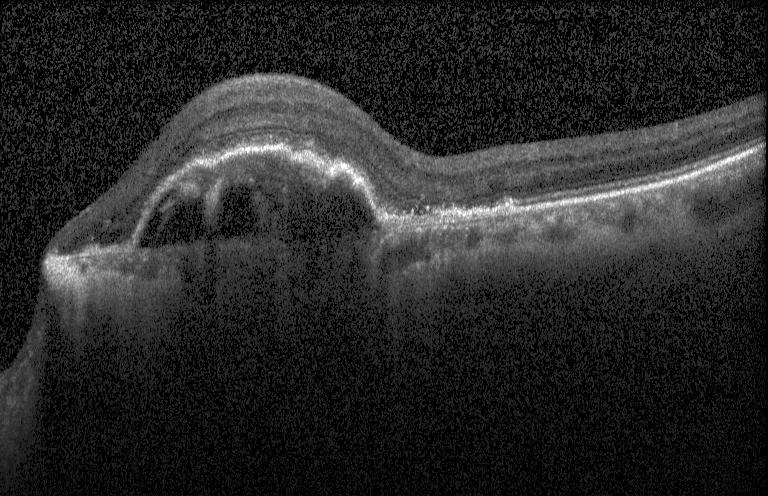

OCT B-scan, instrument: Heidelberg Spectralis, macular scan — The scan shows a choroidal neovascular membrane.